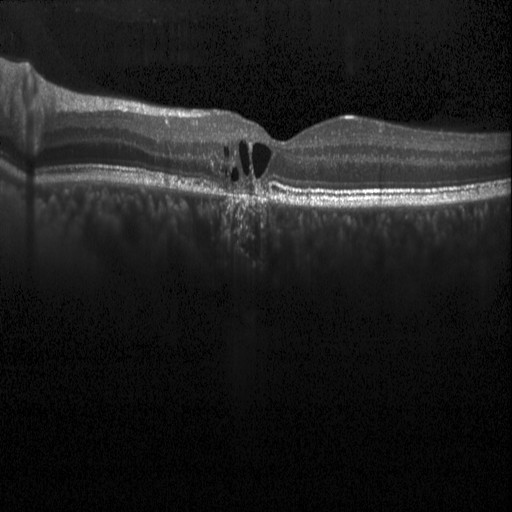
Retinal OCT B-scan. OCT finding: diabetic macular edema.